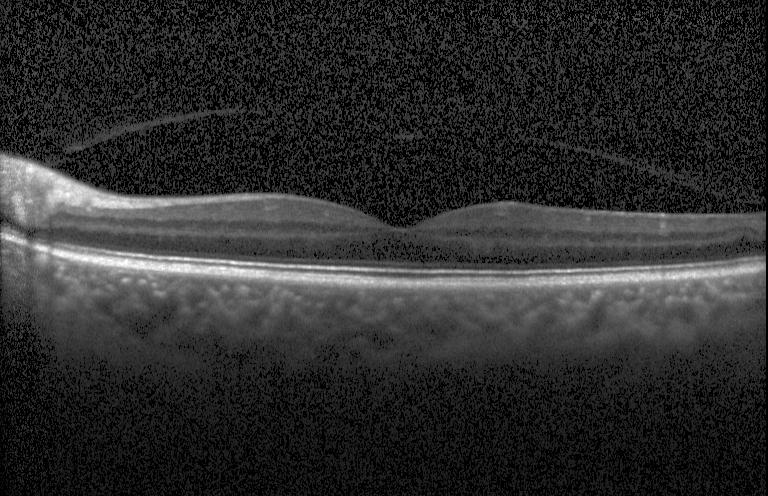
Diagnosis: no evidence of CNV, DME, or drusen.